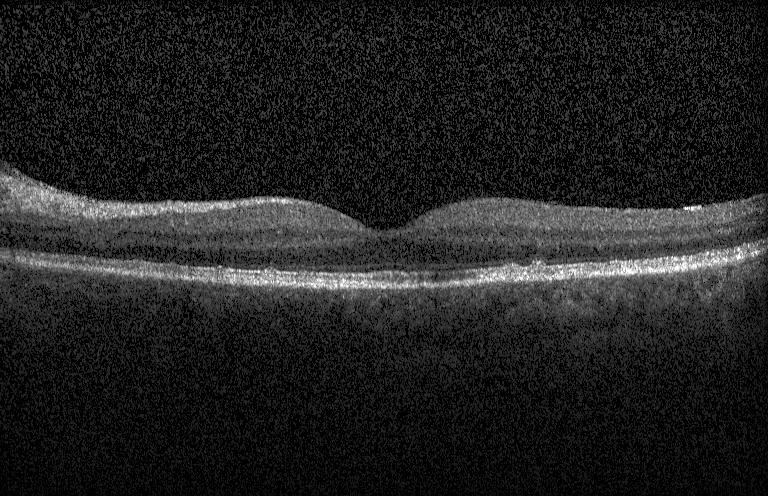
Retinal OCT B-scan. Heidelberg Spectralis. SD-OCT. Through the macula.
Sub-RPE drusenoid deposits.